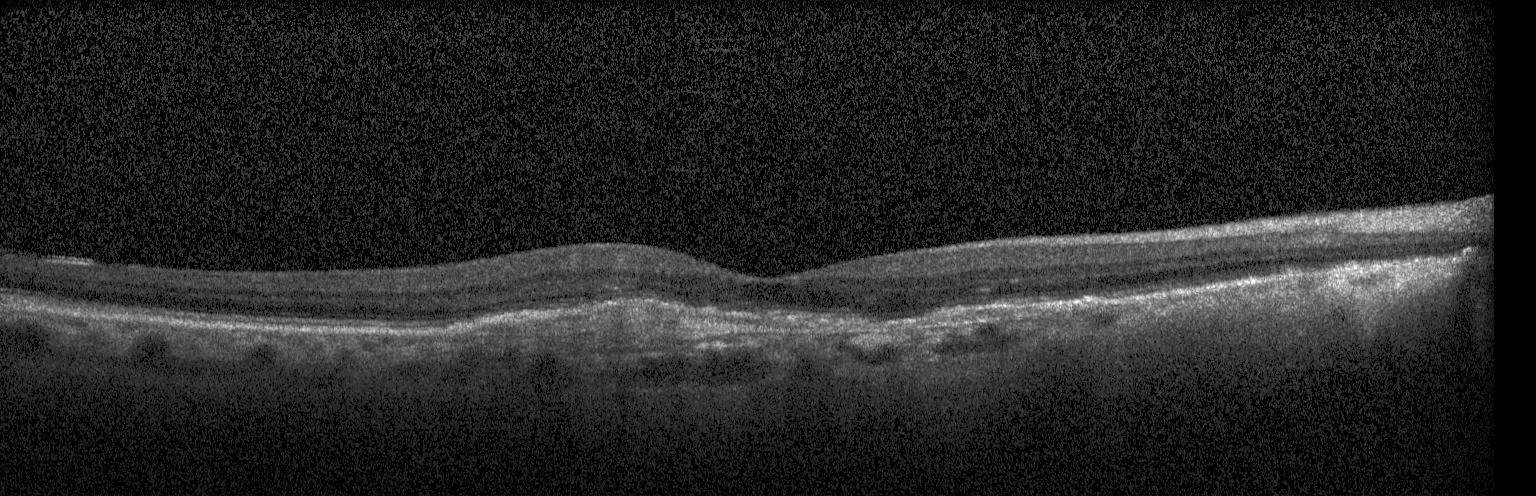 Optical coherence tomography B-scan; spectral-domain optical coherence tomography; macular scan. Diagnosis: a choroidal neovascular membrane.